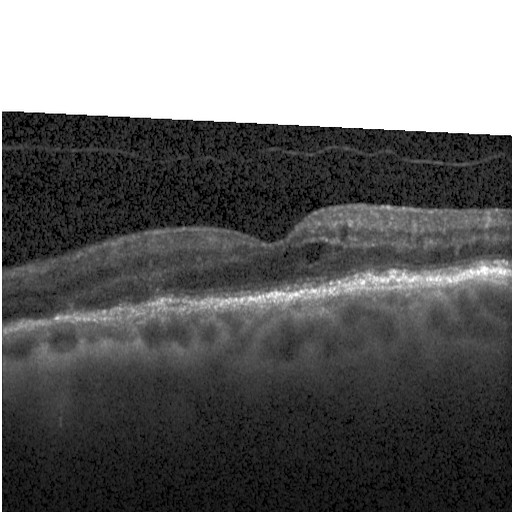
Diagnosis: diabetic macular edema (DME).